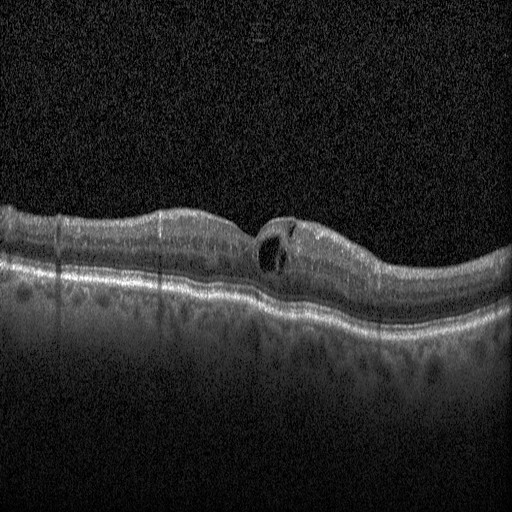 Instrument: Heidelberg Spectralis, macular scan, OCT B-scan. The scan shows DME.